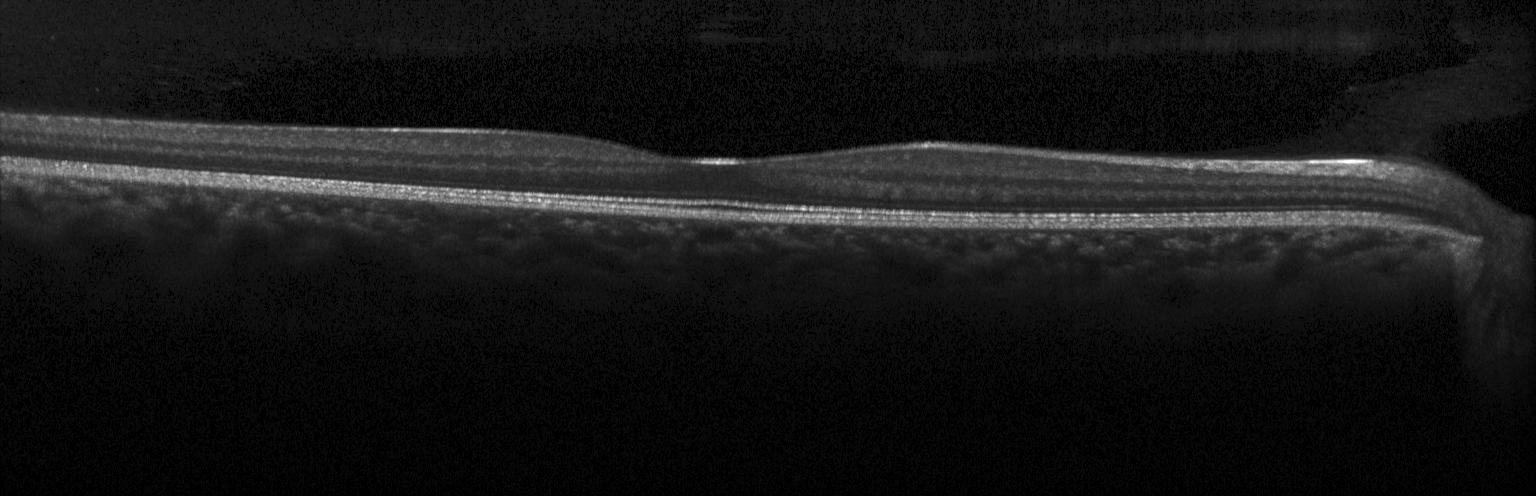
SD-OCT. OCT B-scan. This B-scan demonstrates no CNV, DME, or drusen.